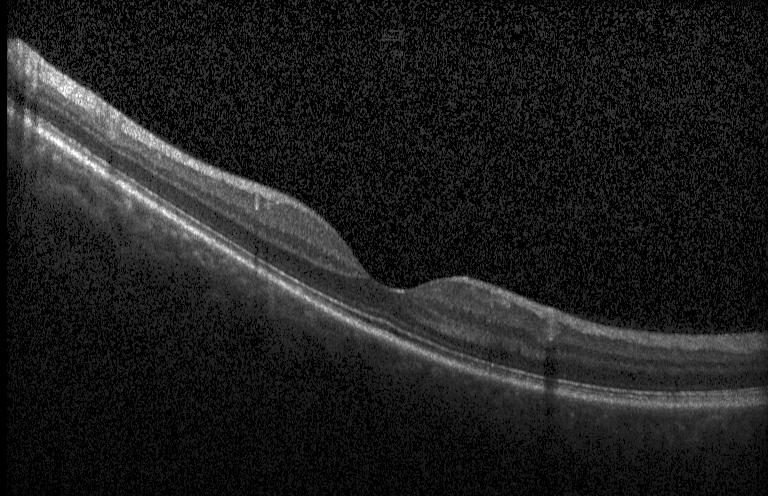

OCT B-scan; acquired on a Heidelberg Spectralis; spectral-domain OCT — Impression: no CNV, DME, or drusen.